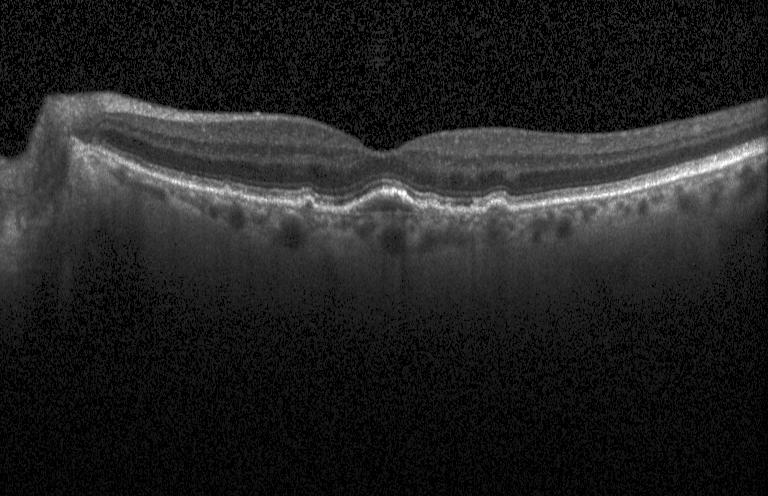

Optical coherence tomography B-scan; macular scan. Impression: a choroidal neovascular membrane.